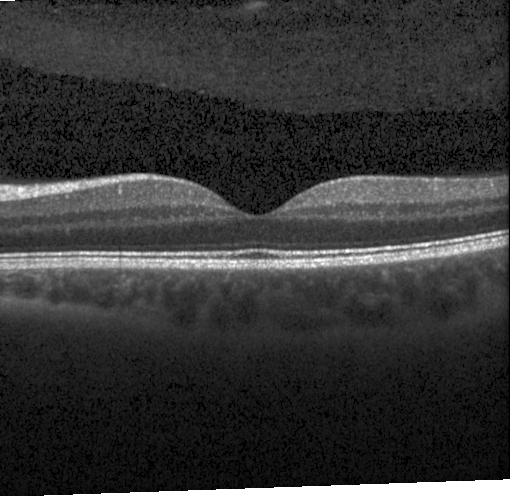

Retinal OCT B-scan. Acquired on a Heidelberg Spectralis. Fovea-centered. No evidence of choroidal neovascularization, diabetic macular edema, or drusen.